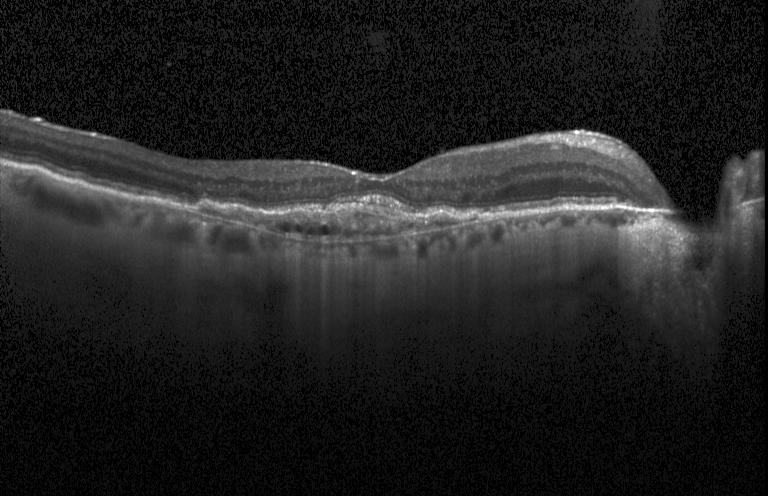

Macular OCT: a choroidal neovascular membrane.